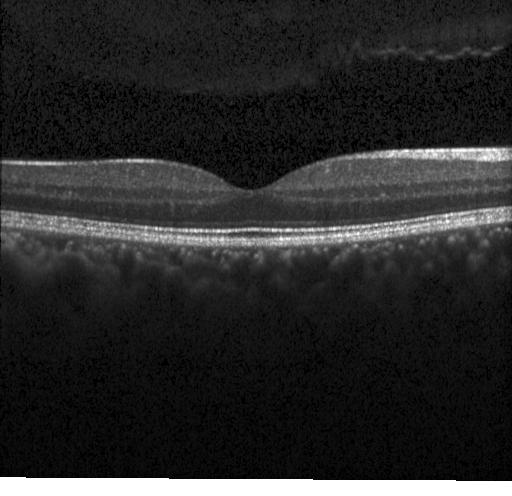

OCT scan showing neither choroidal neovascularization, diabetic macular edema, nor drusen.